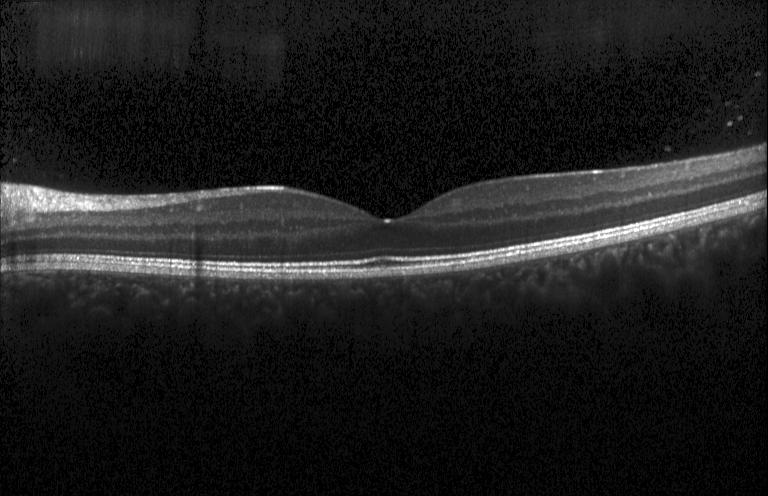
Retinal OCT cross-section — Finding: no CNV, no DME, and no drusen.